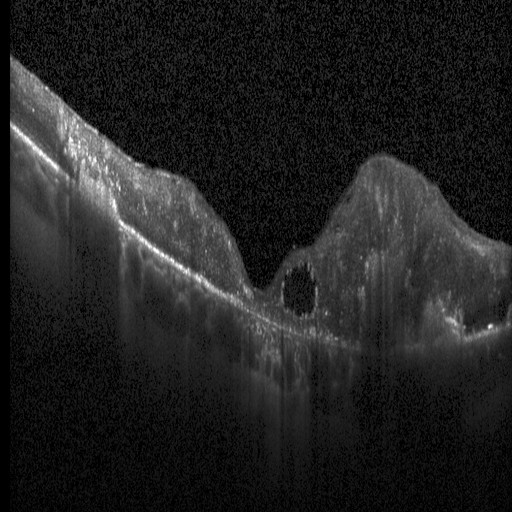
Heidelberg Spectralis OCT system. SD-OCT. OCT line scan
Assessment: diabetic macular edema (DME).